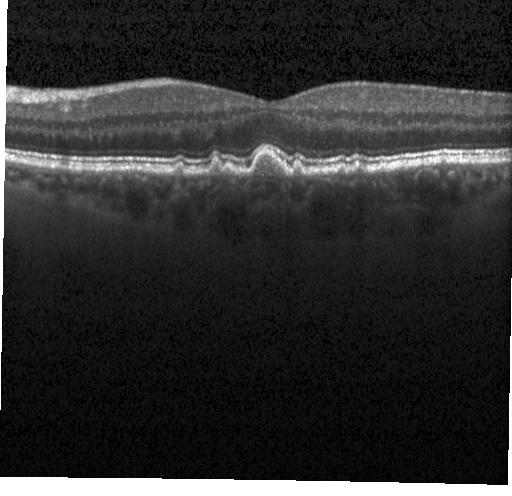 Horizontal scan through the fovea; acquired on a Heidelberg Spectralis; spectral-domain optical coherence tomography; optical coherence tomography B-scan.
Finding: multiple drusen.